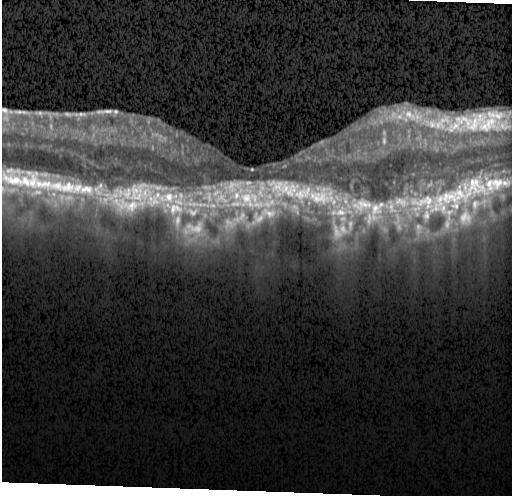

OCT line scan · fovea-centered · Heidelberg Spectralis · spectral-domain OCT. Diagnosis: choroidal neovascularization.